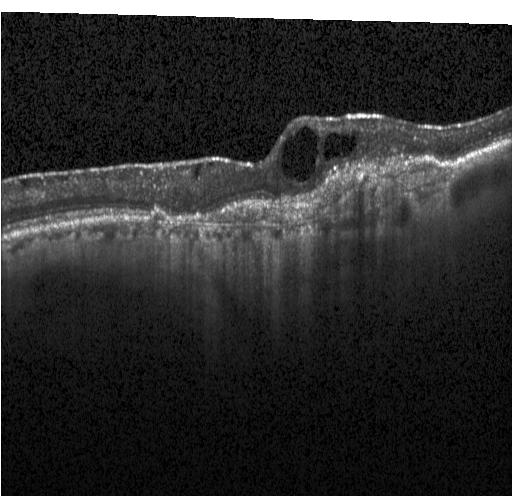 Centered on the fovea. Spectral-domain optical coherence tomography. Retinal OCT B-scan. A choroidal neovascular membrane.